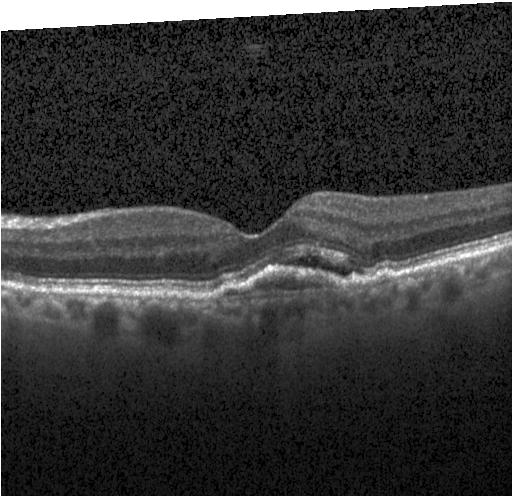

Finding: choroidal neovascularization.